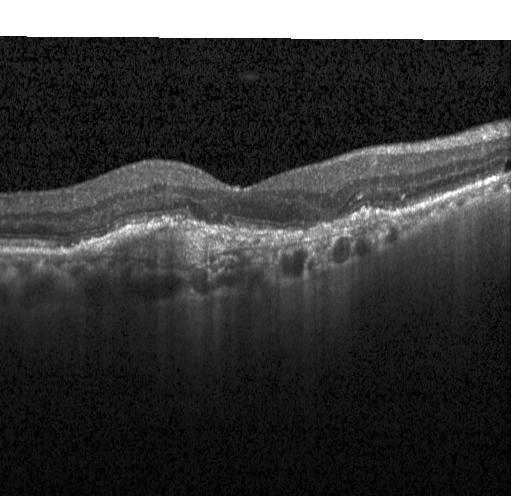 The scan shows choroidal neovascularization (CNV).